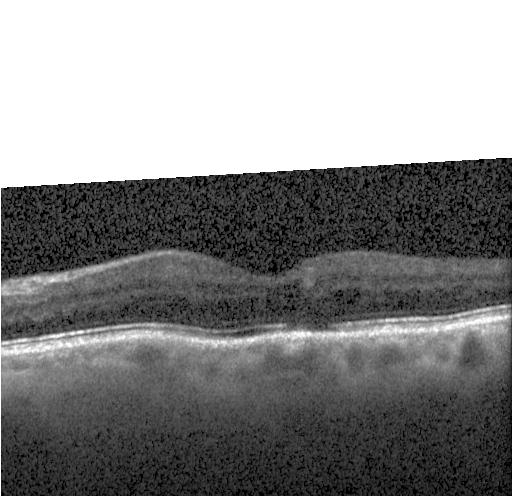

Finding: neither choroidal neovascularization, diabetic macular edema, nor drusen.